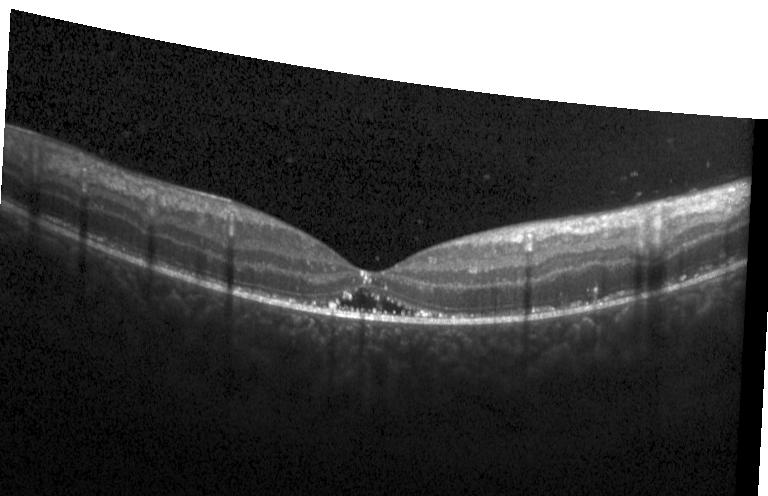

Assessment: a choroidal neovascular membrane.